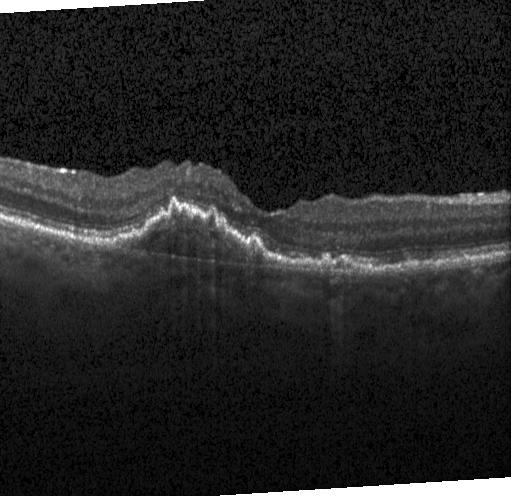

Retinal OCT cross-section showing choroidal neovascularization (CNV).